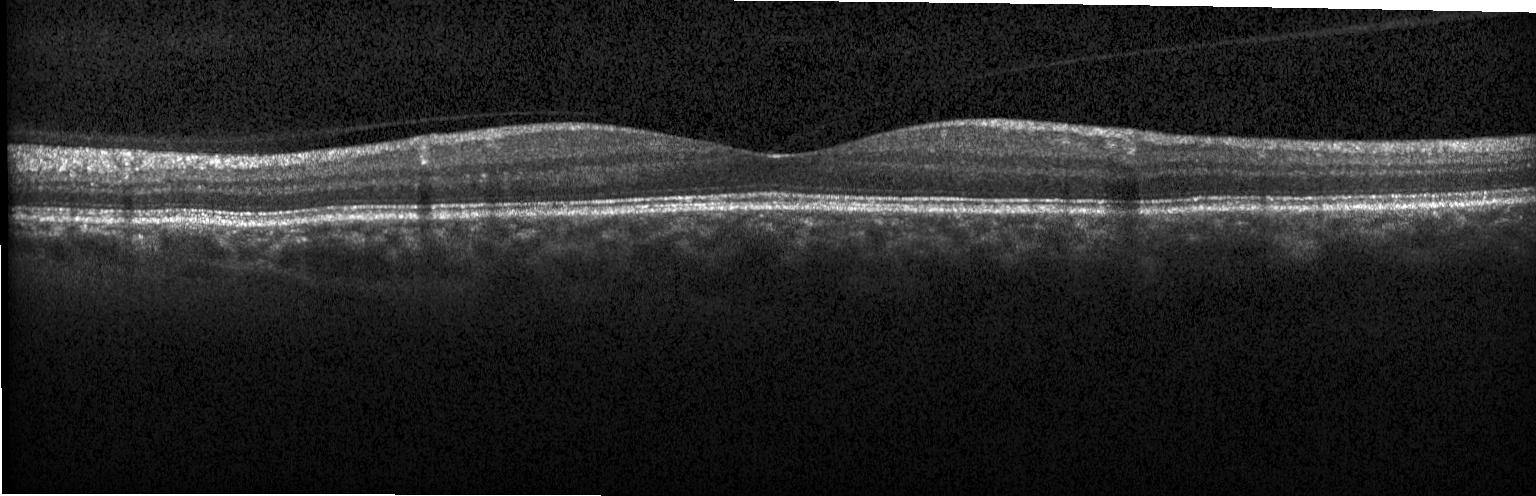
OCT finding: neither choroidal neovascularization, diabetic macular edema, nor drusen.